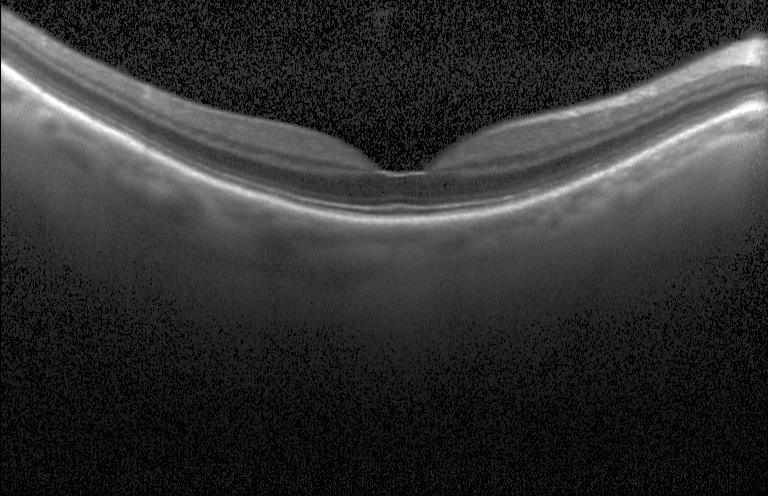
Impression: no choroidal neovascularization, diabetic macular edema, or drusen.